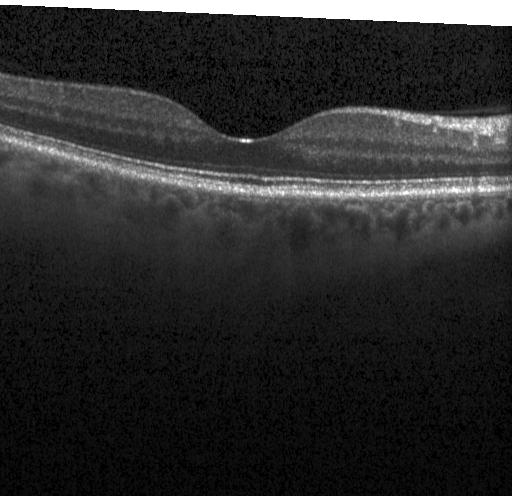 Fovea-centered. Heidelberg Spectralis. Retinal OCT B-scan. SD-OCT — The scan shows neither CNV, DME, nor drusen.